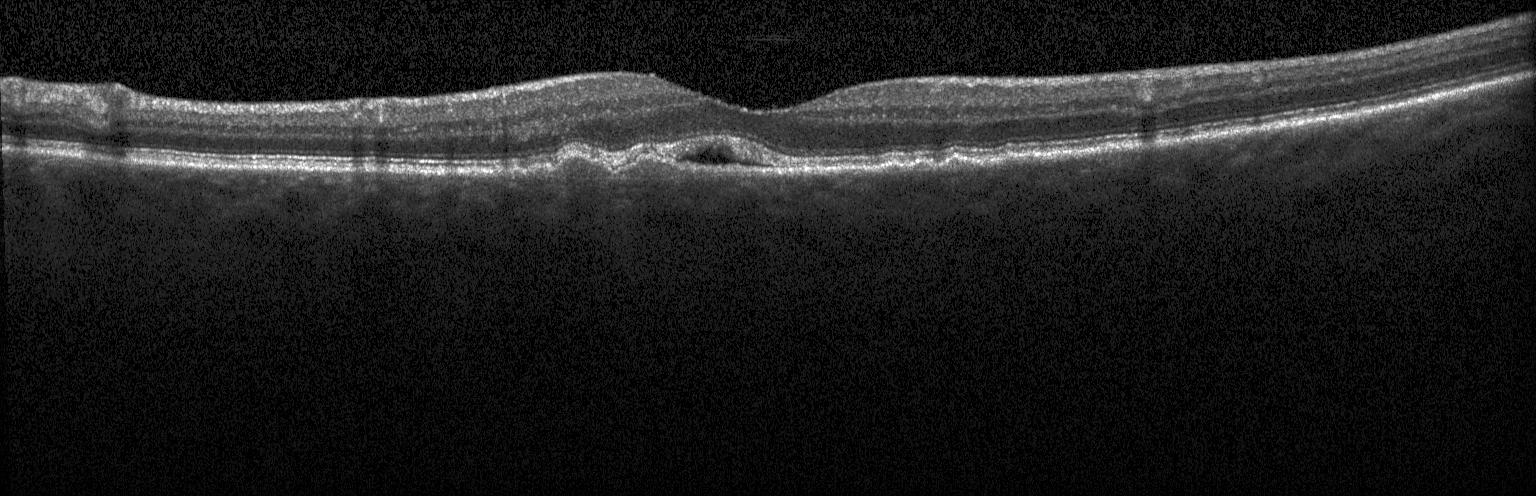

Heidelberg Spectralis OCT system · retinal OCT cross-section · spectral-domain OCT · fovea-centered — Finding: a choroidal neovascular membrane.